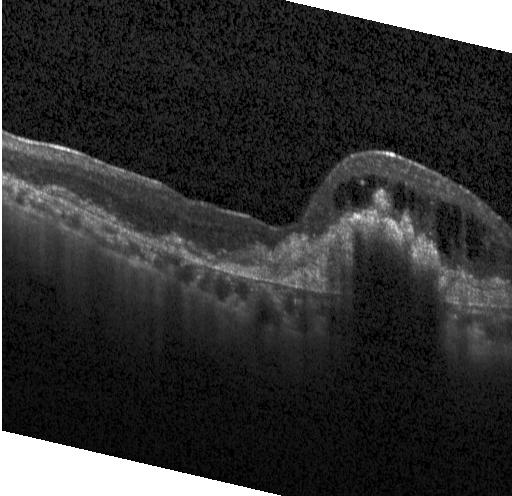 Macular OCT: a choroidal neovascular membrane.